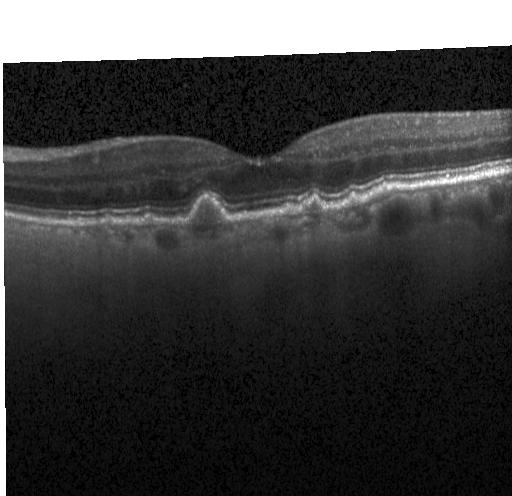 Spectral-domain OCT; OCT B-scan; Heidelberg Spectralis OCT system; macular scan
Assessment: drusen.